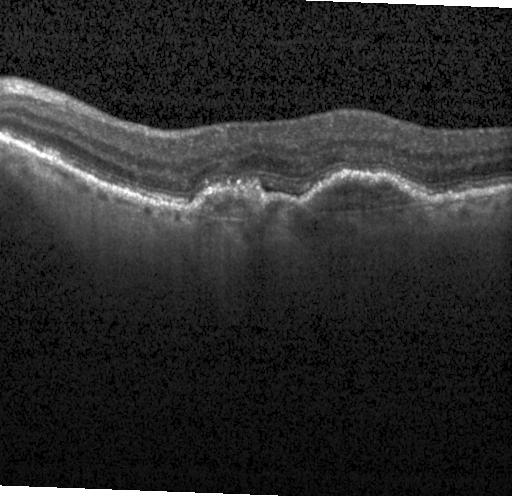

Impression: a choroidal neovascular membrane.